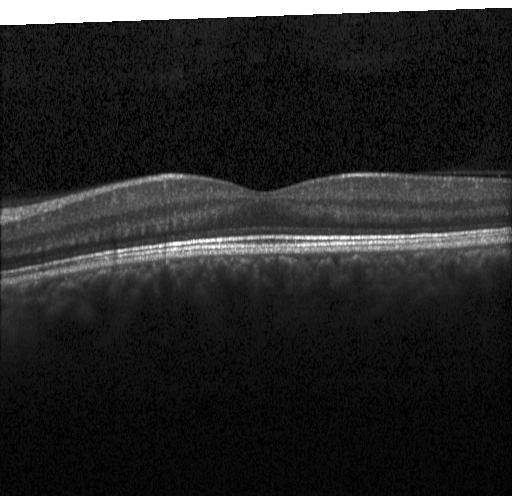
OCT B-scan; spectral-domain optical coherence tomography; centered on the fovea. Diagnosis: no CNV, no DME, and no drusen.